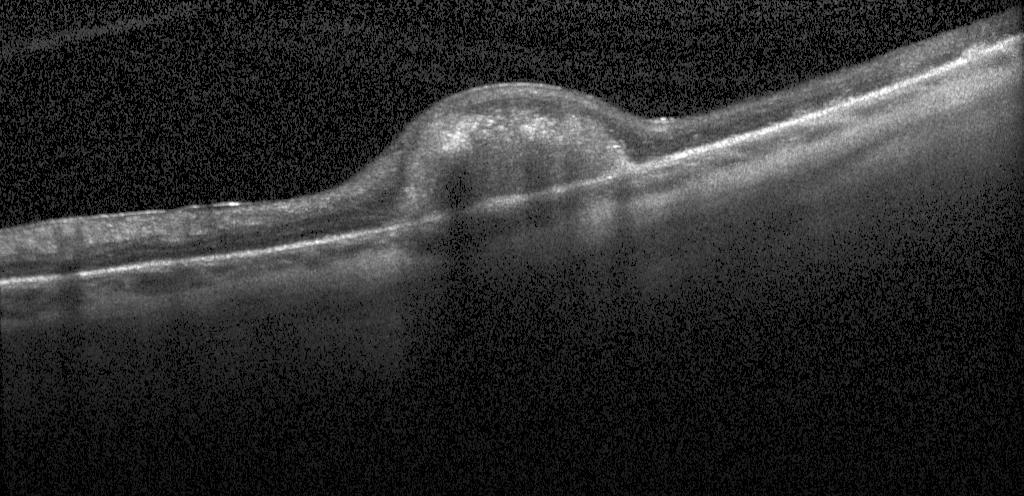
OCT B-scan; spectral-domain optical coherence tomography; macular scan — A choroidal neovascular membrane.